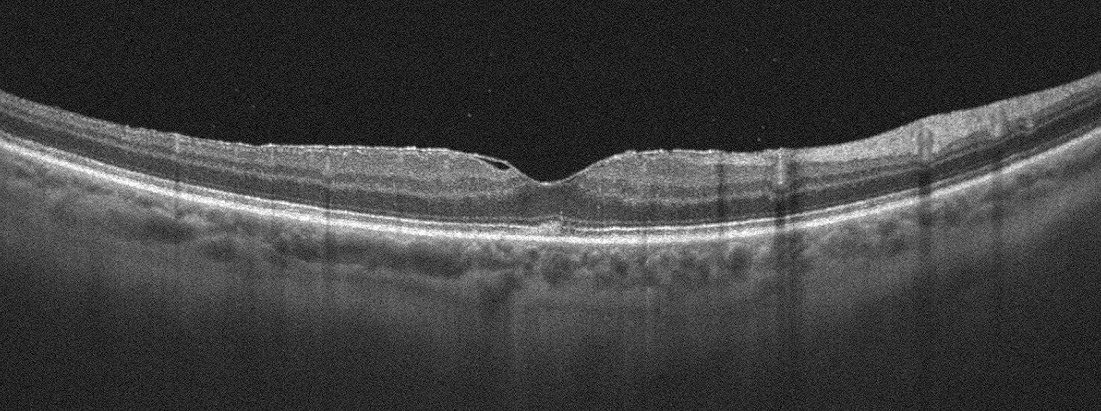
This B-scan demonstrates ERM.